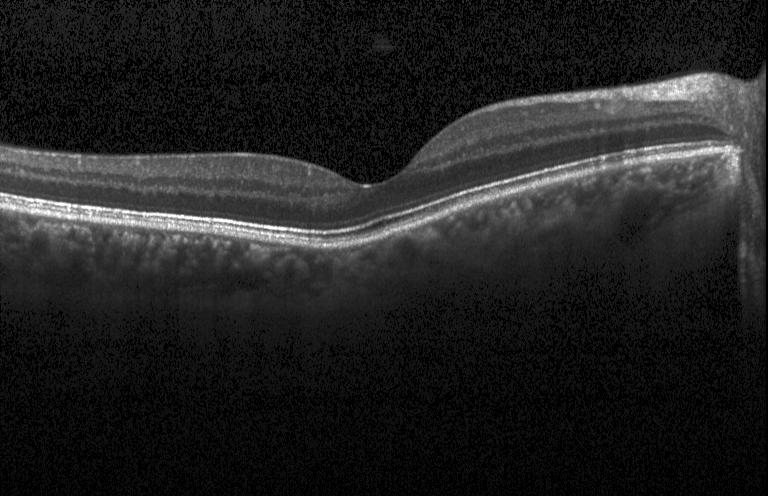

Retinal OCT B-scan — OCT finding: no evidence of CNV, DME, or drusen.